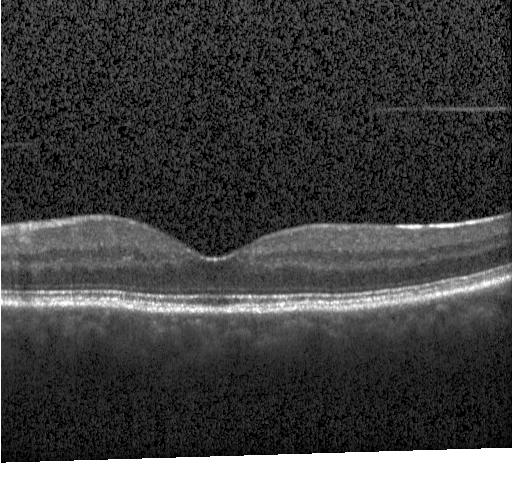
Impression: no choroidal neovascularization, no diabetic macular edema, and no drusen.